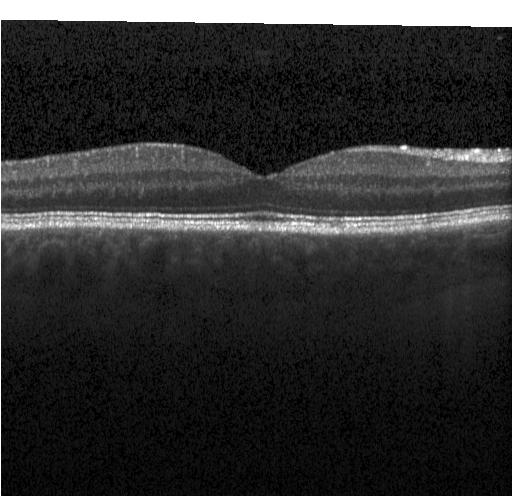

Retinal OCT cross-section showing no choroidal neovascularization, diabetic macular edema, or drusen.